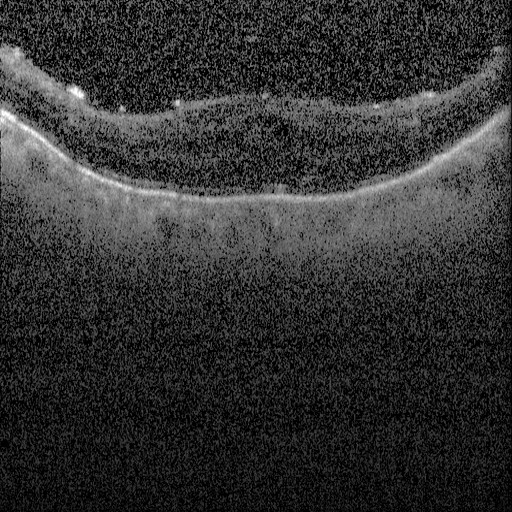 Diagnosis: diabetic macular edema (DME).